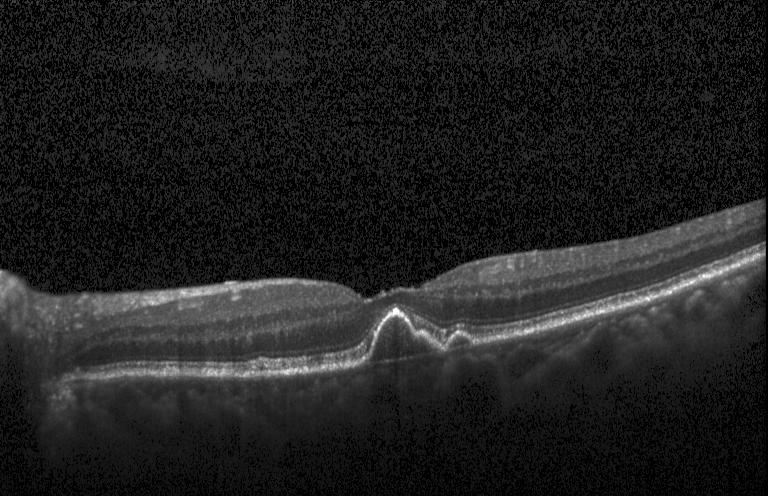 Retinal OCT B-scan.
Finding: a choroidal neovascular membrane.